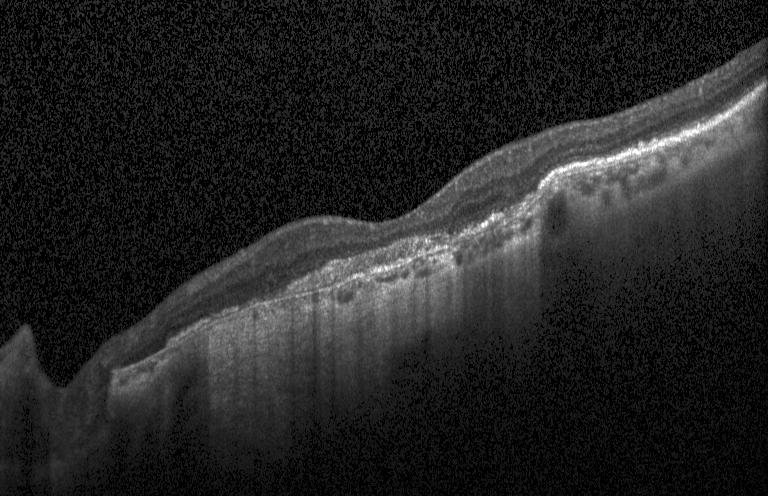
Retinal OCT B-scan. Diagnosis: a choroidal neovascular membrane.